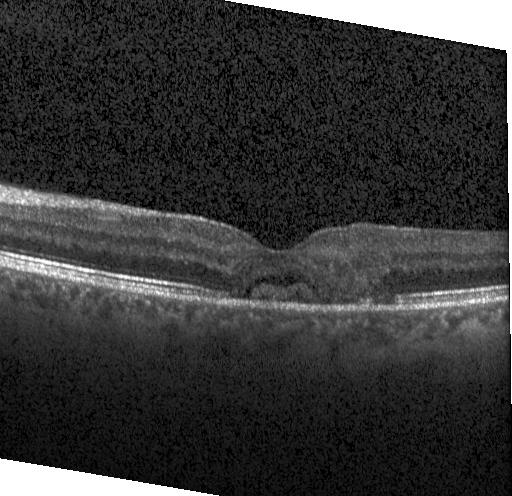
Spectral-domain OCT · optical coherence tomography B-scan. Impression: CNV.